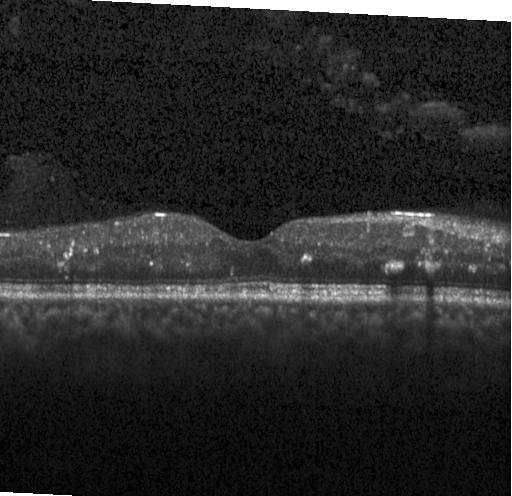 Diagnosis: diabetic macular edema.